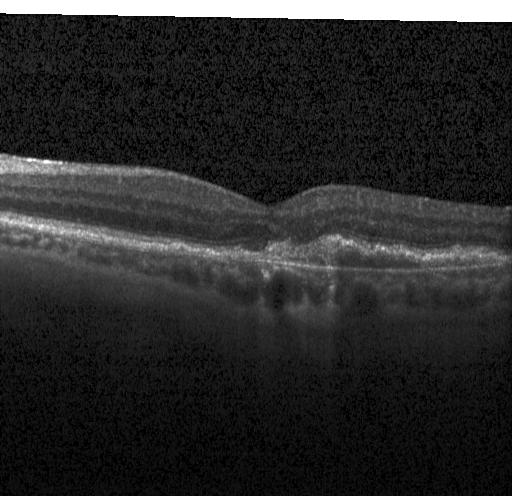
Dx: a choroidal neovascular membrane.